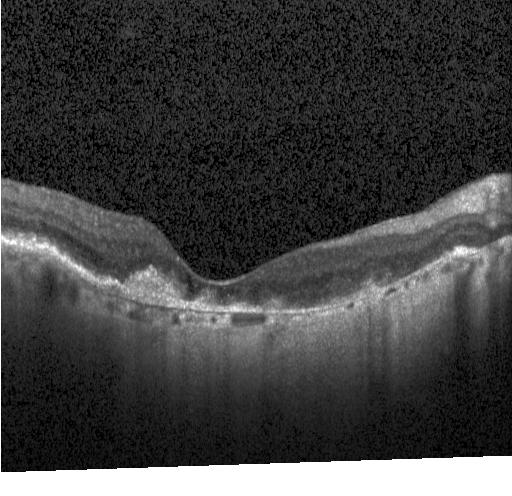

OCT B-scan; Heidelberg Spectralis OCT system — Impression: a choroidal neovascular membrane.